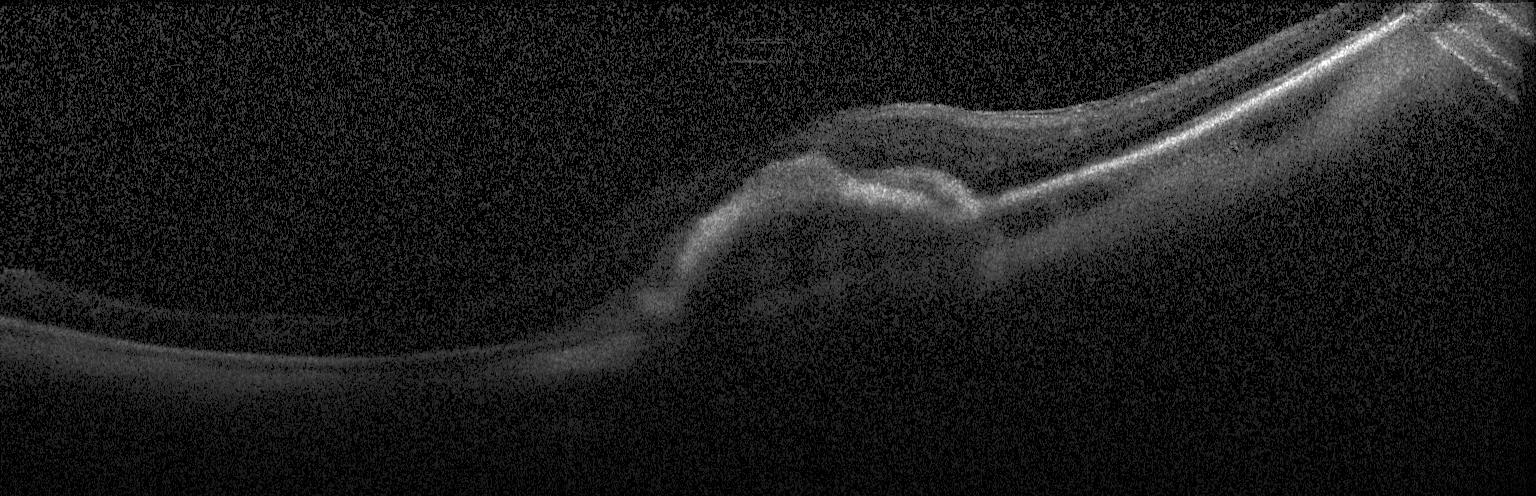 Acquired on a Heidelberg Spectralis · macular scan · retinal OCT cross-section · spectral-domain optical coherence tomography
OCT finding: choroidal neovascularization.